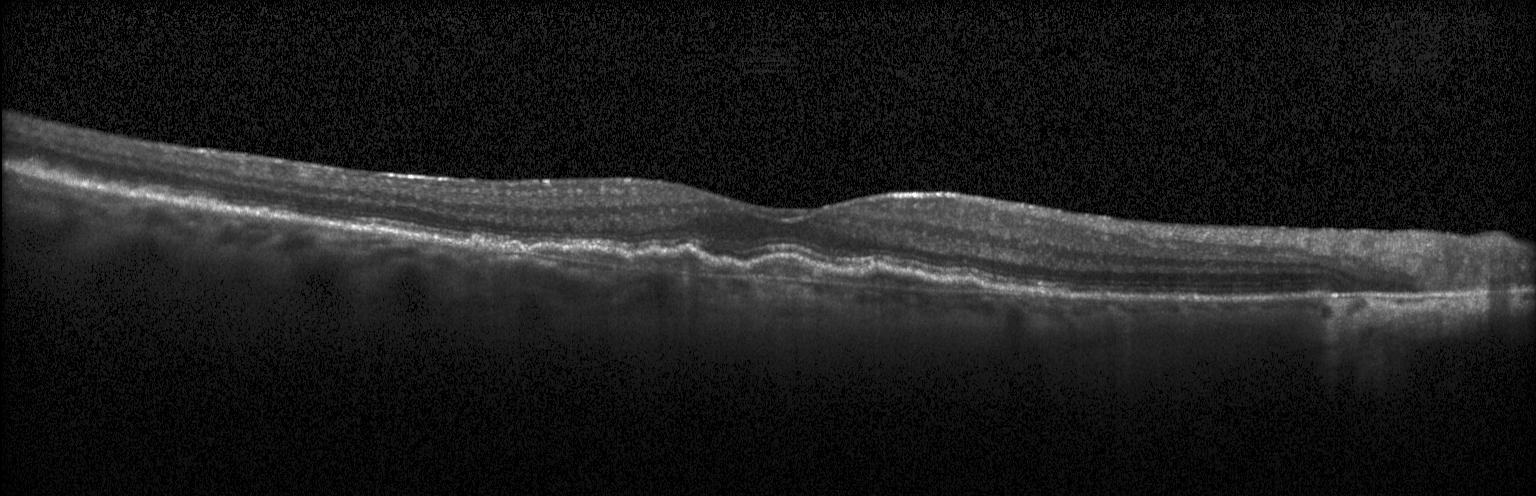

Finding: choroidal neovascularization (CNV).